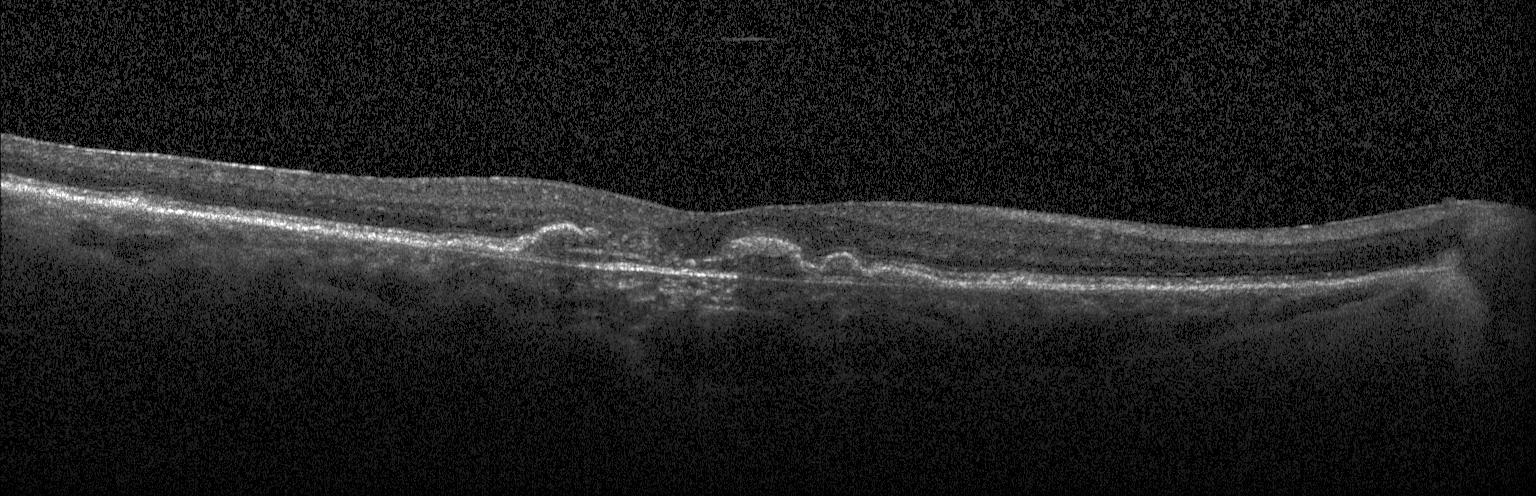

Retinal OCT cross-section, Heidelberg Spectralis OCT system, spectral-domain optical coherence tomography, through the macula
Impression: choroidal neovascularization.